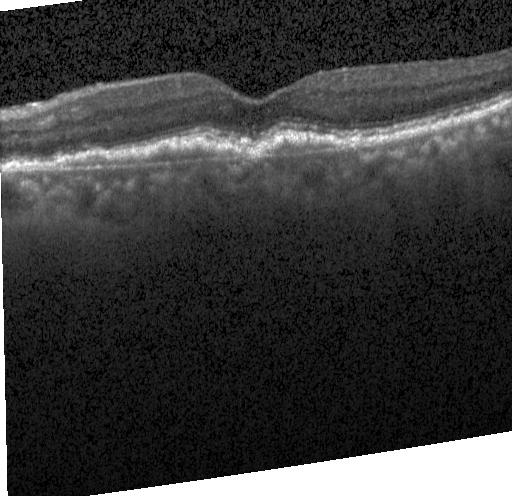
OCT B-scan — Diagnosis: CNV.